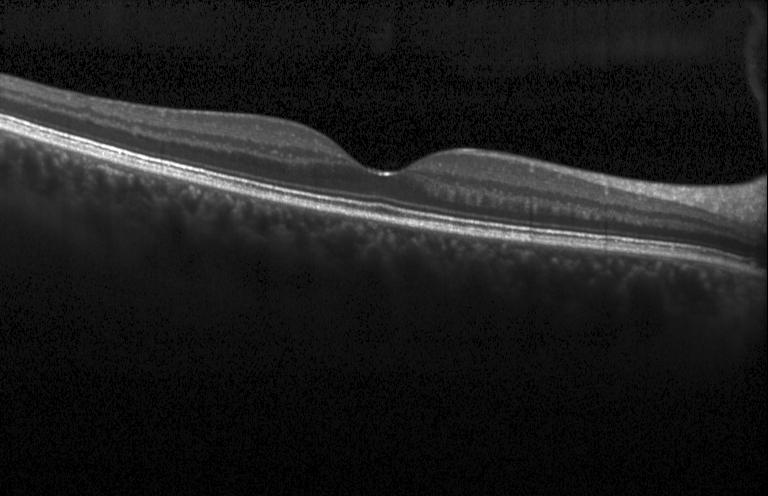
Macular scan · OCT B-scan · SD-OCT · acquired on a Heidelberg Spectralis.
Impression: neither choroidal neovascularization, diabetic macular edema, nor drusen.